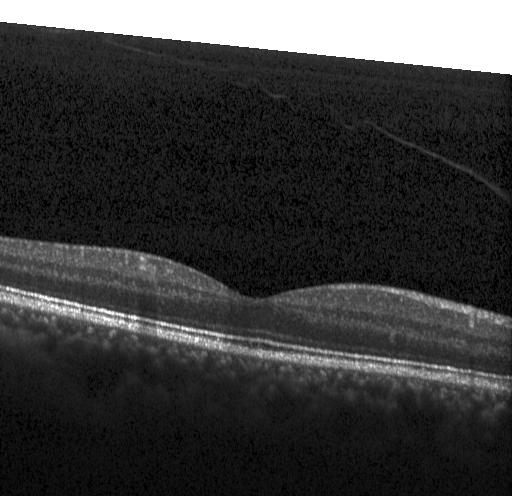 The scan shows no CNV, DME, or drusen.